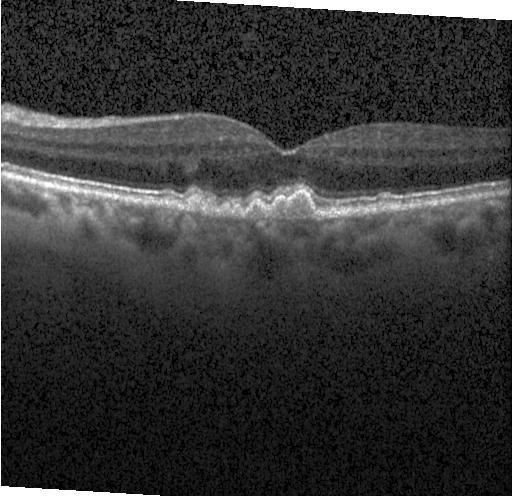

Retinal OCT B-scan
This B-scan demonstrates drusen.